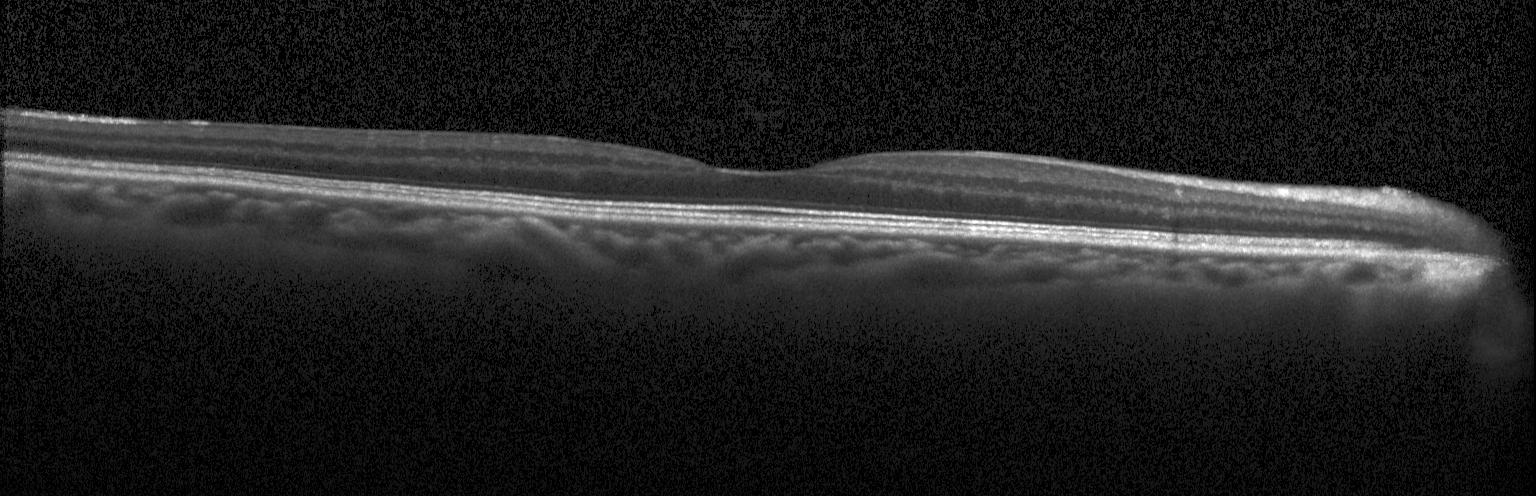 OCT finding: neither choroidal neovascularization, diabetic macular edema, nor drusen.